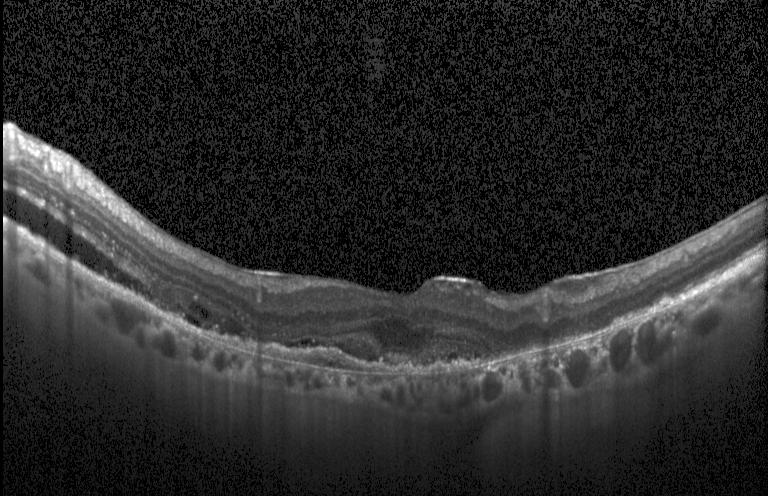 OCT B-scan.
Diagnosis: choroidal neovascularization.